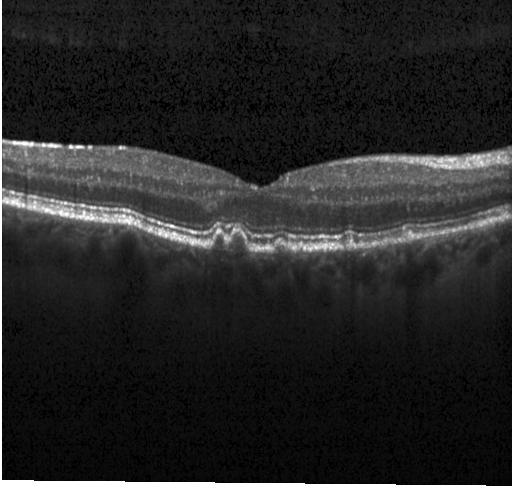

Macular OCT: sub-RPE drusenoid deposits.